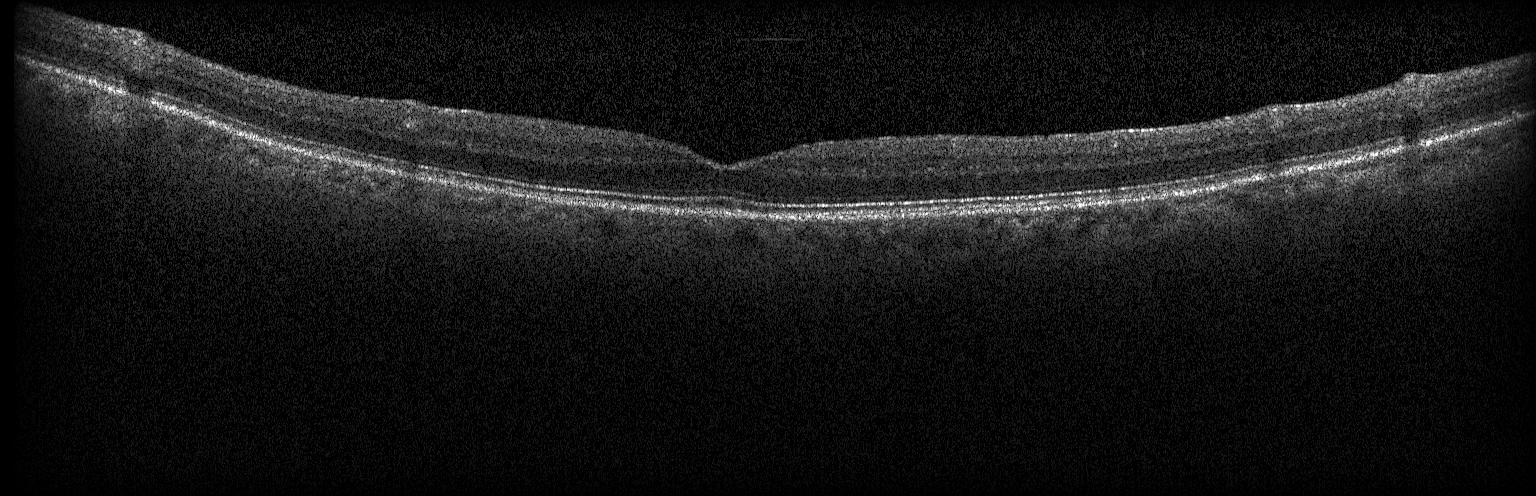 OCT line scan · spectral-domain OCT · horizontal scan through the fovea
Diagnosis: neither choroidal neovascularization, diabetic macular edema, nor drusen.